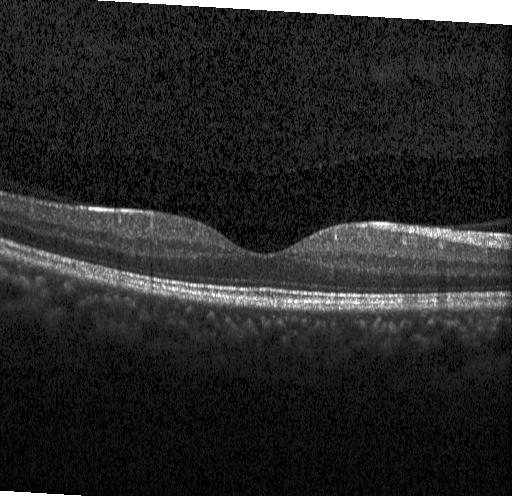

OCT line scan. Acquired on a Heidelberg Spectralis. Centered on the fovea. SD-OCT
Impression: no evidence of CNV, DME, or drusen.